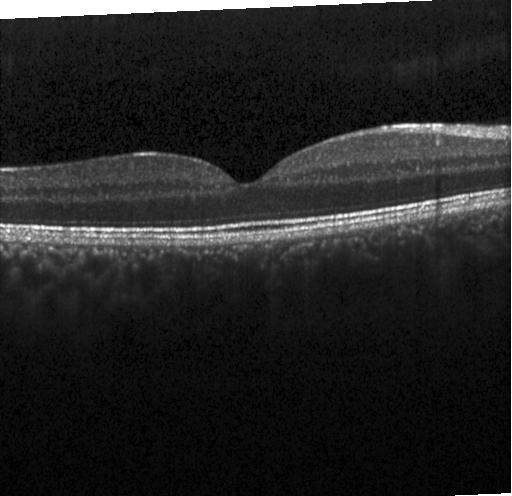
Retinal OCT cross-section showing no choroidal neovascularization, no diabetic macular edema, and no drusen.